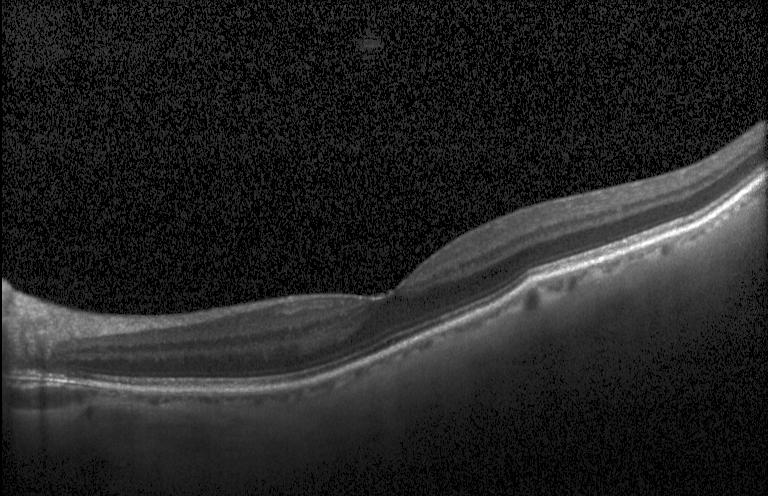

OCT B-scan — The scan shows neither CNV, DME, nor drusen.